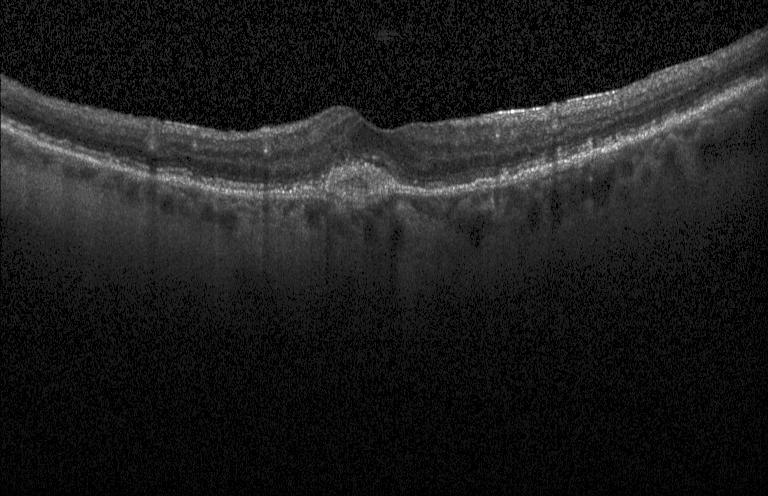 Spectral-domain OCT · OCT B-scan · horizontal scan through the fovea — CNV.